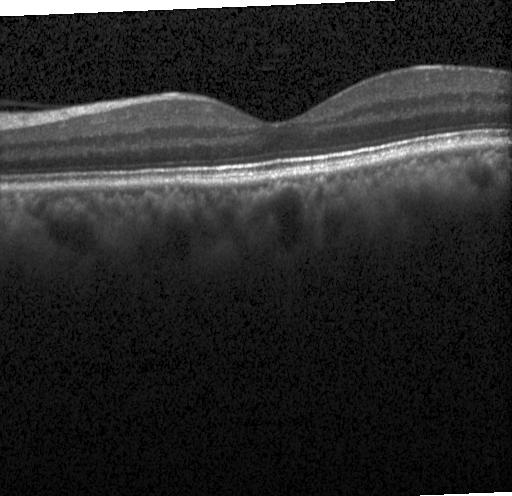

Diagnosis: neither choroidal neovascularization, diabetic macular edema, nor drusen.